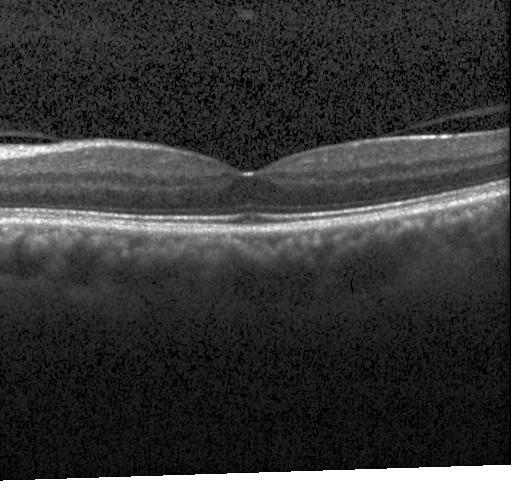

Dx: no choroidal neovascularization, diabetic macular edema, or drusen.